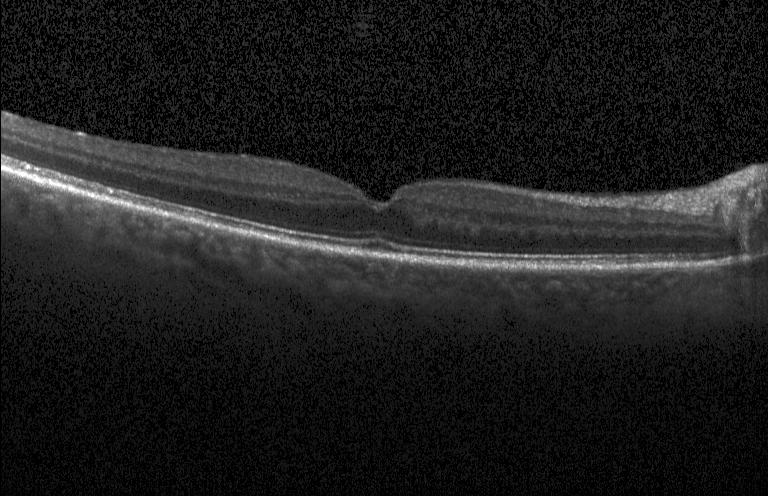
OCT B-scan showing no CNV, DME, or drusen.